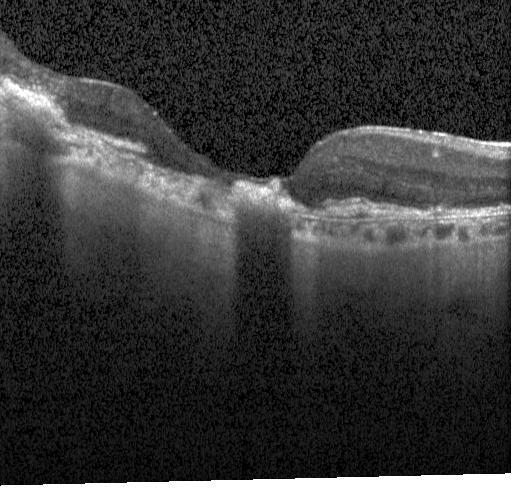

Instrument: Heidelberg Spectralis. Spectral-domain optical coherence tomography. Retinal OCT B-scan — Assessment: CNV.